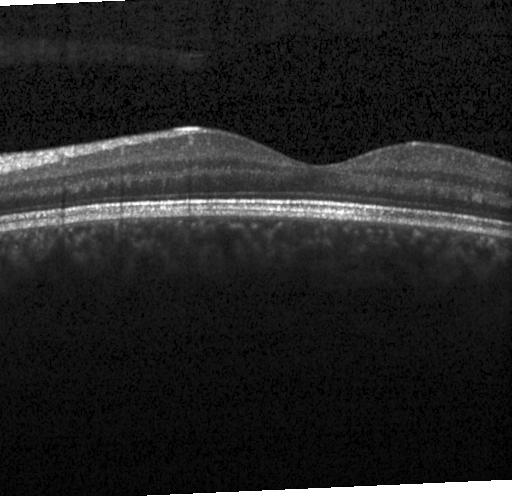
Retinal OCT cross-section showing no evidence of choroidal neovascularization, diabetic macular edema, or drusen.